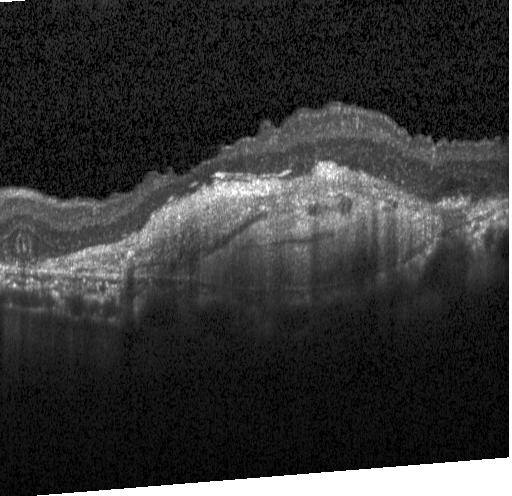
OCT B-scan. Finding: a choroidal neovascular membrane.